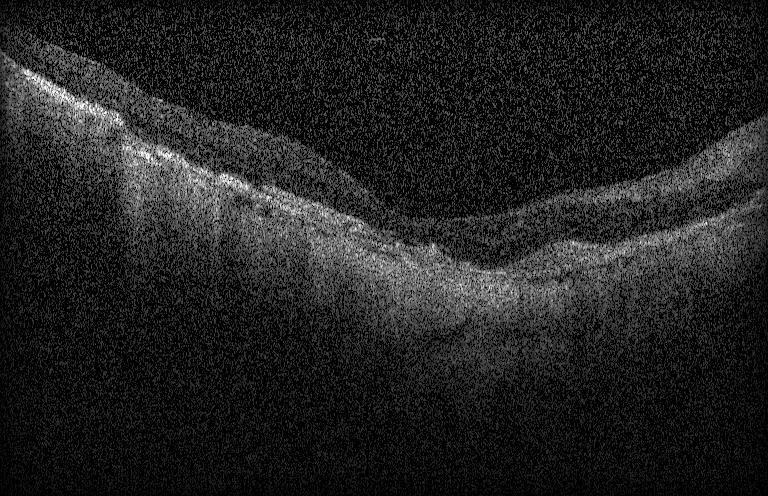
OCT scan showing a choroidal neovascular membrane.